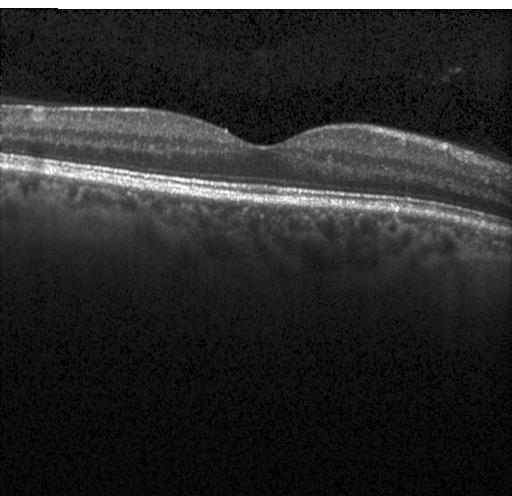
Centered on the fovea; OCT line scan — Impression: no choroidal neovascularization, no diabetic macular edema, and no drusen.